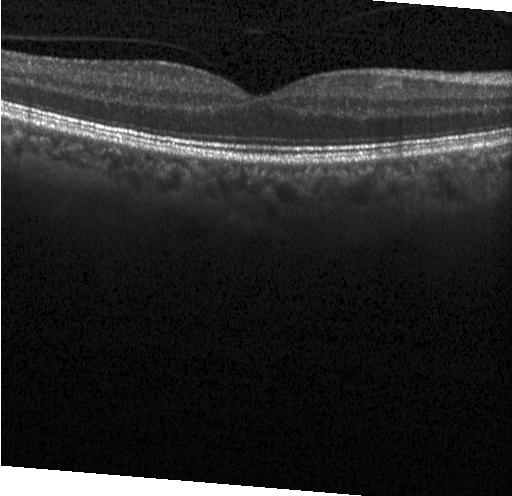 This B-scan demonstrates no CNV, DME, or drusen.